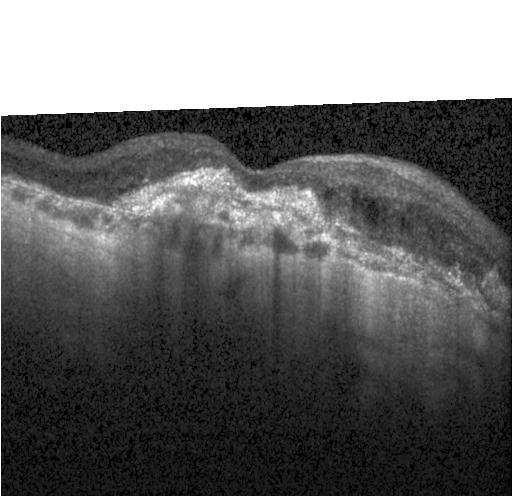
OCT line scan — Diagnosis: CNV.